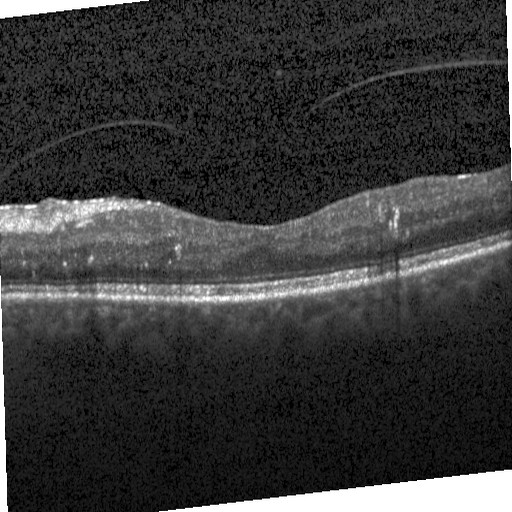 Spectral-domain optical coherence tomography. Retinal OCT cross-section. Through the macula. Instrument: Heidelberg Spectralis — Finding: diabetic macular edema (DME).